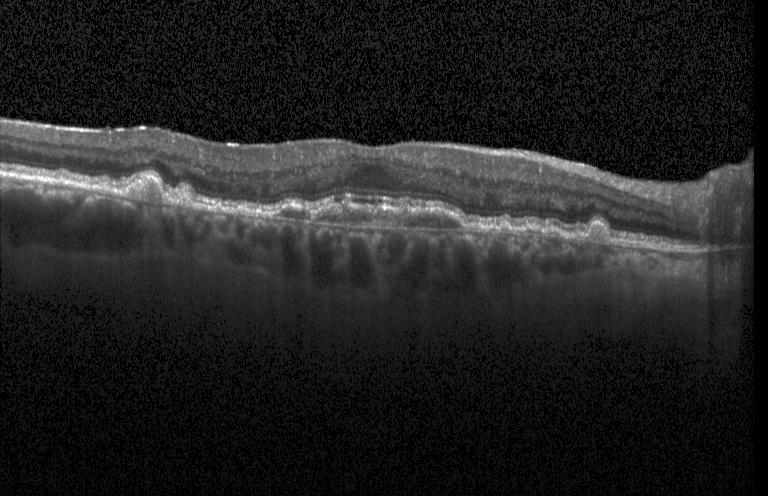 OCT finding: a choroidal neovascular membrane.